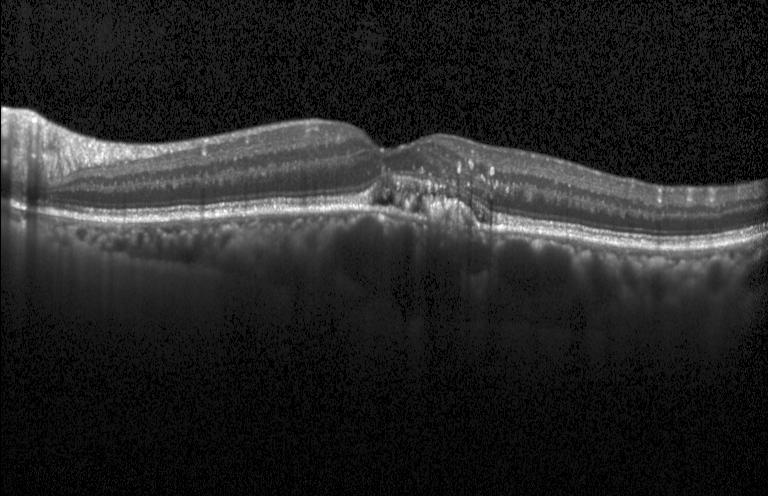
Optical coherence tomography scan.
The scan shows choroidal neovascularization (CNV).